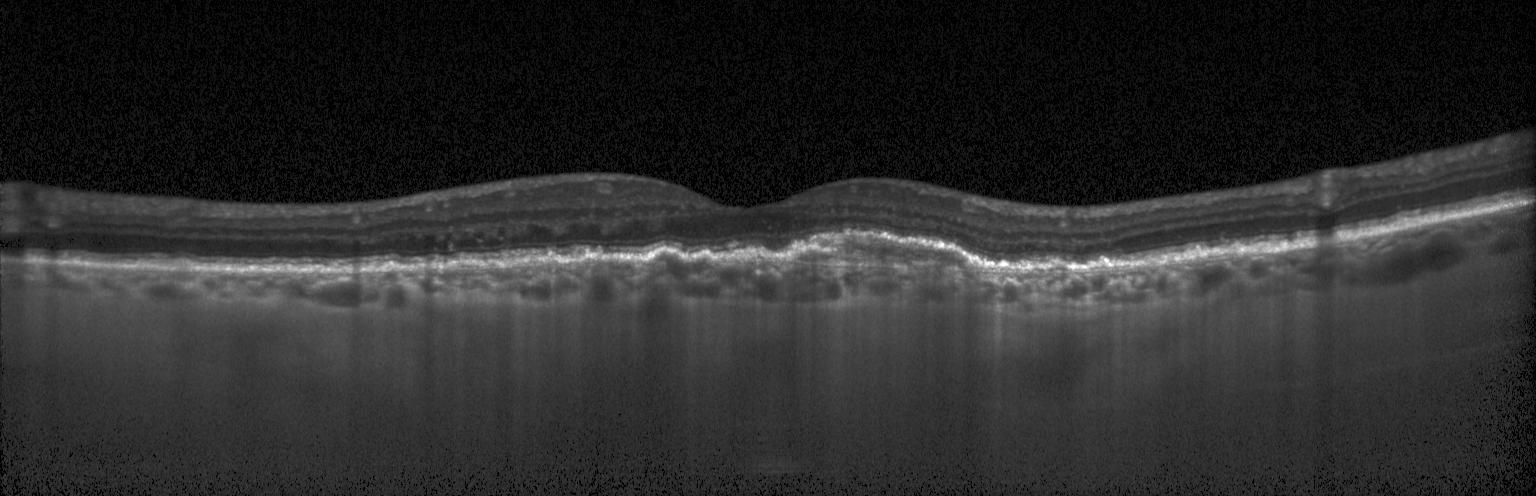 The scan shows choroidal neovascularization (CNV).